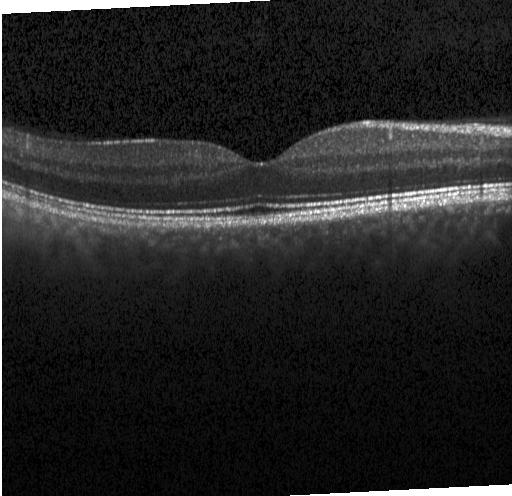
Heidelberg Spectralis OCT system. Retinal OCT B-scan — Assessment: no CNV, DME, or drusen.